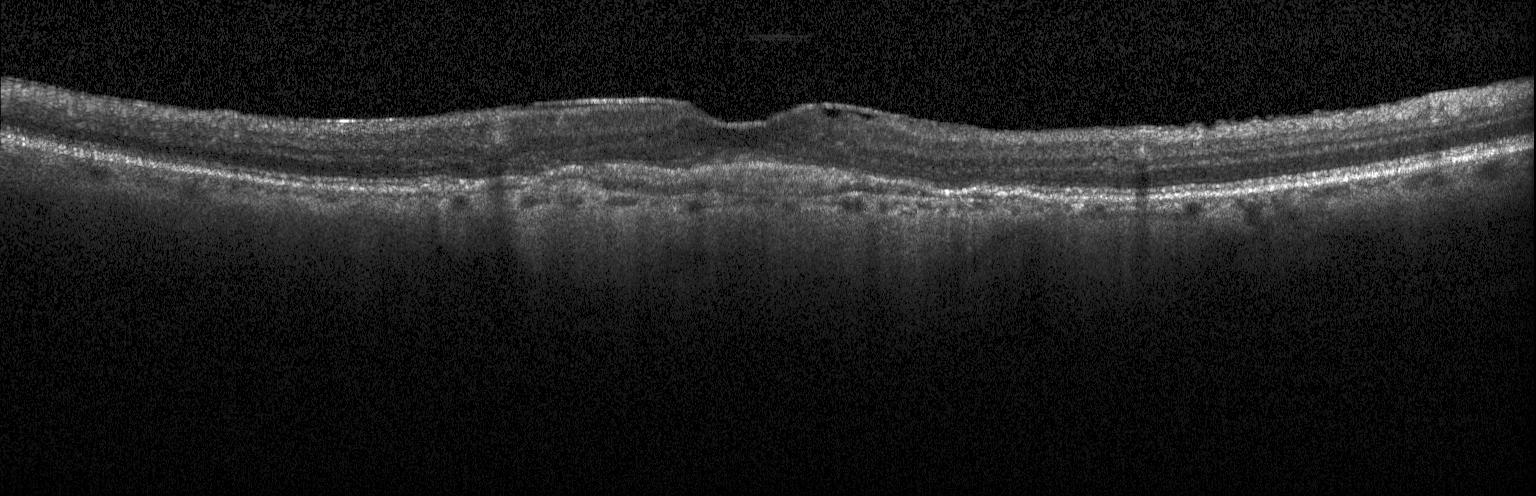

Dx: a choroidal neovascular membrane.